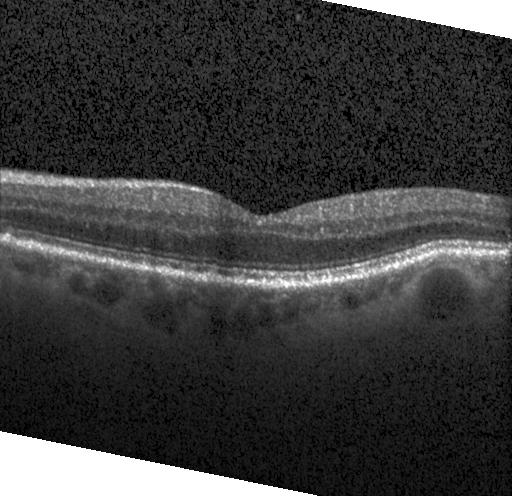
Optical coherence tomography B-scan.
The scan shows no choroidal neovascularization, diabetic macular edema, or drusen.